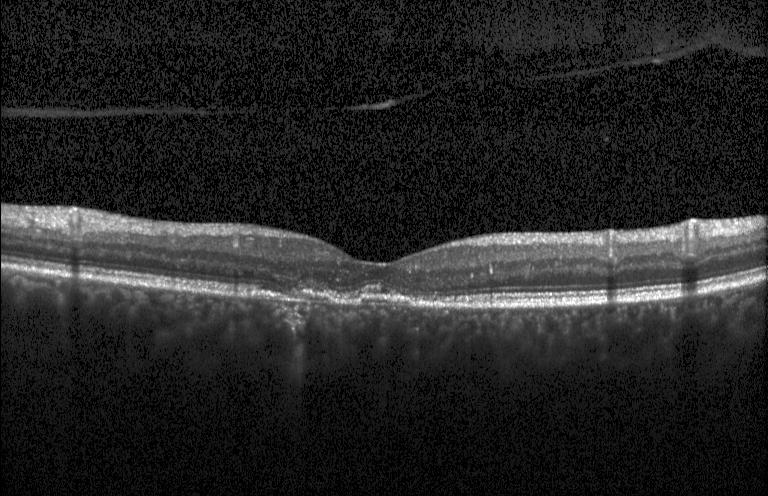

Assessment: a choroidal neovascular membrane.